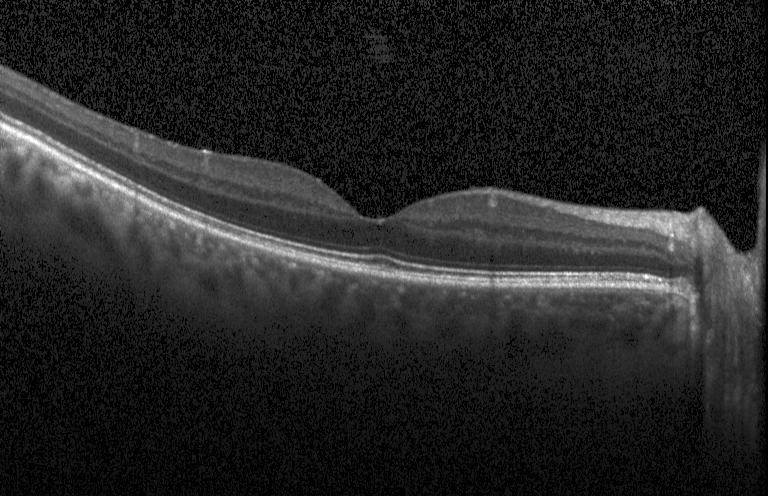
Retinal OCT cross-section; instrument: Heidelberg Spectralis
Impression: no evidence of choroidal neovascularization, diabetic macular edema, or drusen.